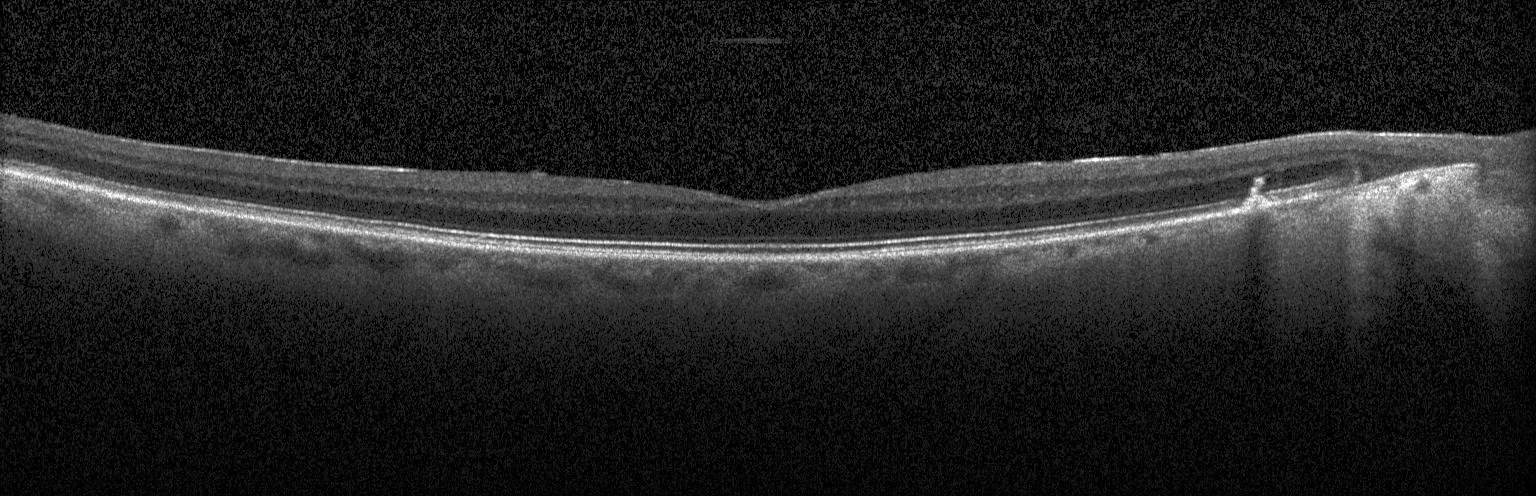

Spectral-domain optical coherence tomography · OCT line scan · instrument: Heidelberg Spectralis.
Diagnosis: no choroidal neovascularization, no diabetic macular edema, and no drusen.